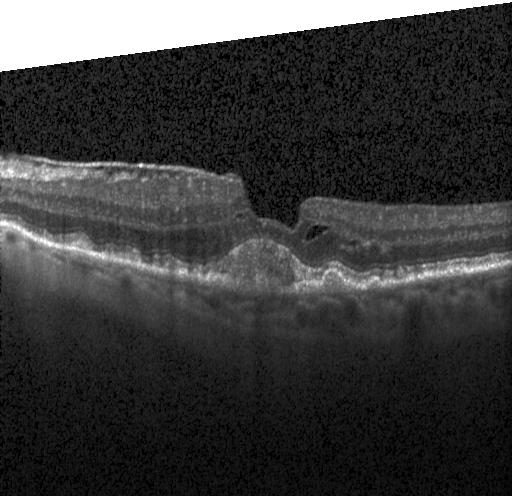 OCT line scan; centered on the fovea. The scan shows a choroidal neovascular membrane.